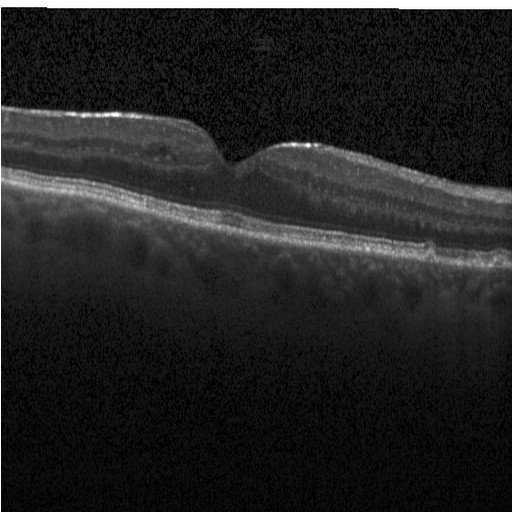

Impression: diabetic macular edema.